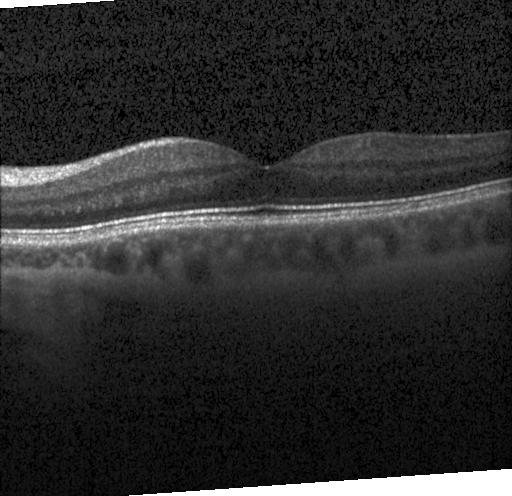

OCT B-scan showing neither CNV, DME, nor drusen.